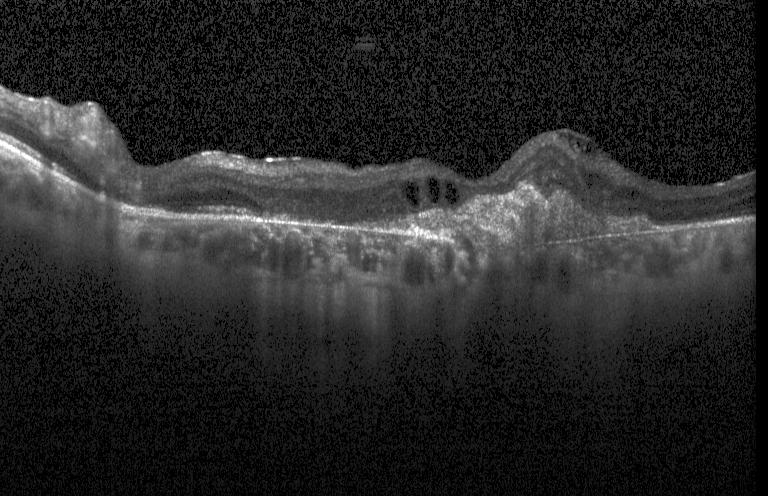

OCT finding: a choroidal neovascular membrane.